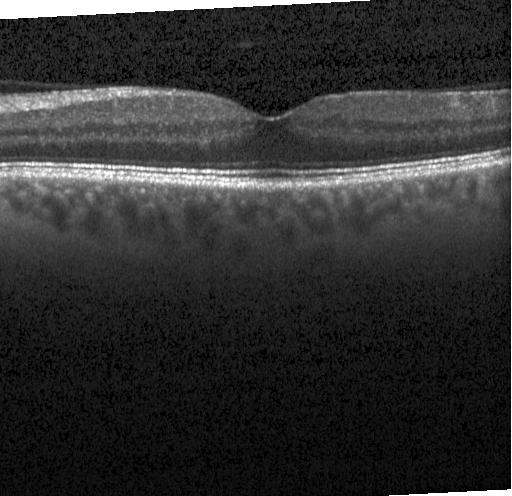 Spectral-domain OCT; optical coherence tomography B-scan; acquired on a Heidelberg Spectralis; centered on the fovea
Finding: no CNV, no DME, and no drusen.